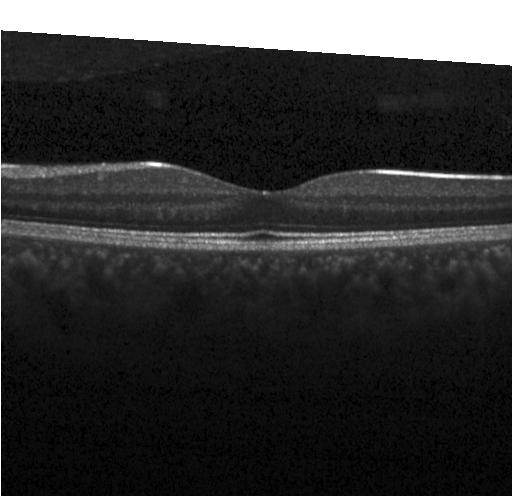

Finding: no choroidal neovascularization, diabetic macular edema, or drusen.